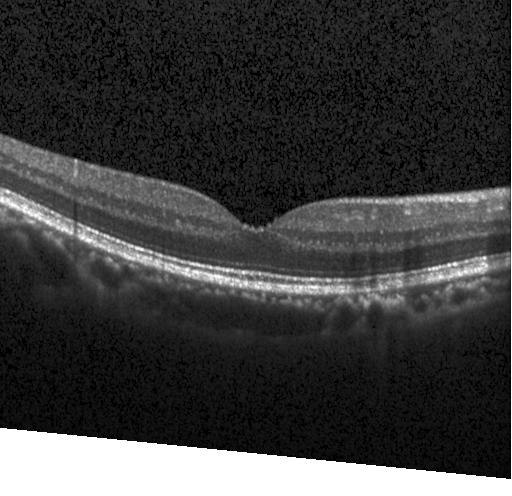
Optical coherence tomography B-scan, horizontal scan through the fovea, spectral-domain optical coherence tomography — This B-scan demonstrates no choroidal neovascularization, no diabetic macular edema, and no drusen.